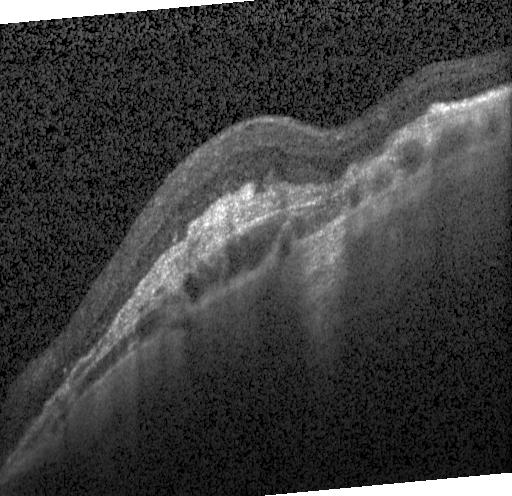
Spectral-domain OCT B-scan: choroidal neovascularization.